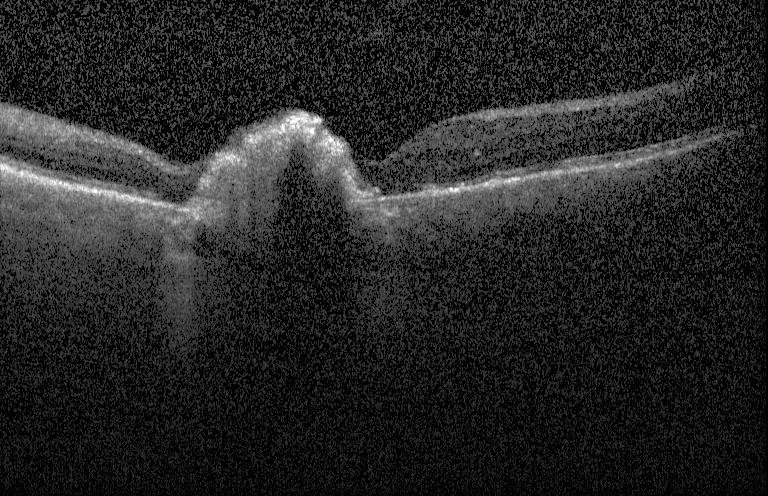 Horizontal scan through the fovea. Optical coherence tomography B-scan
Assessment: choroidal neovascularization.